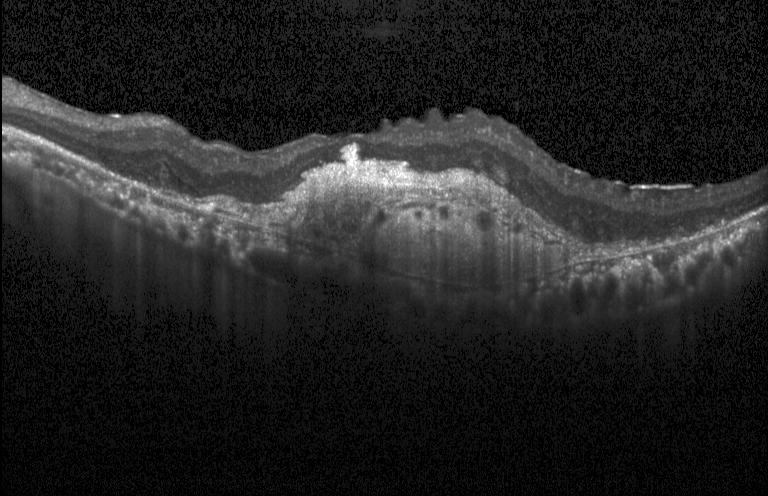 This B-scan demonstrates CNV.